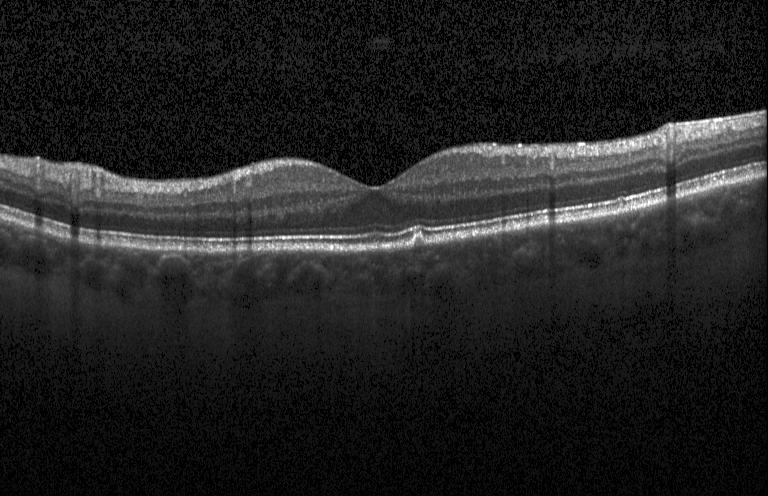

Macular OCT: multiple drusen.